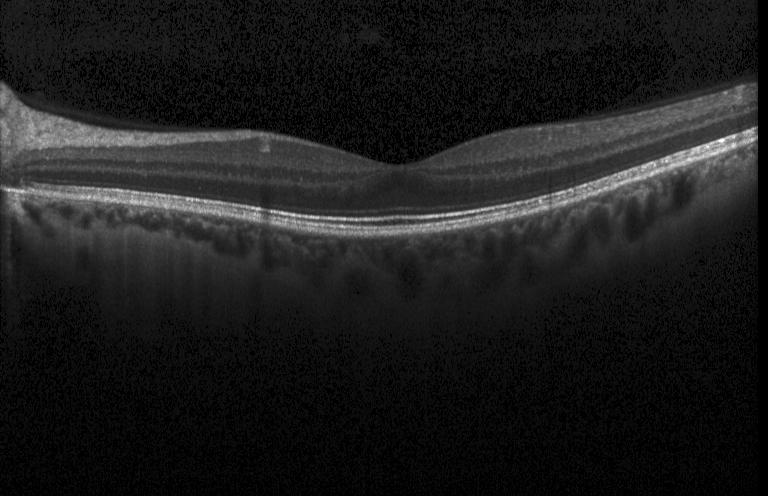 OCT finding: no CNV, DME, or drusen.